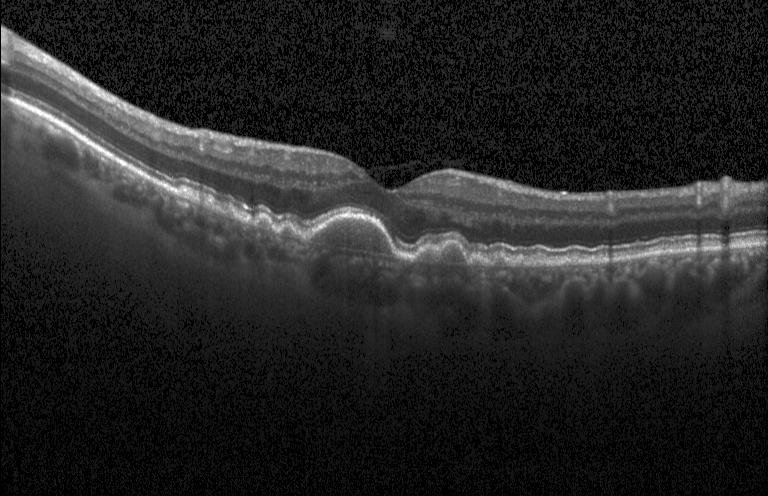 Impression: drusen.